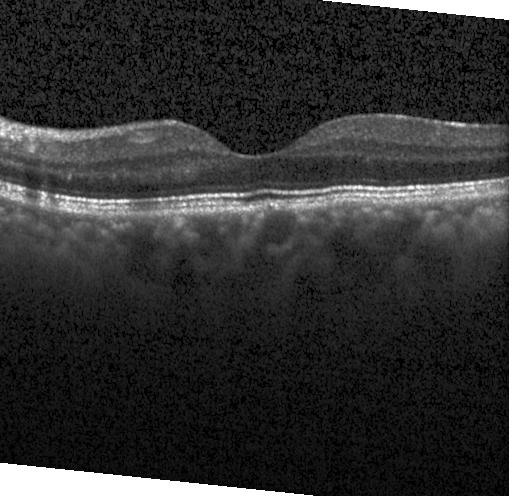

OCT B-scan showing neither CNV, DME, nor drusen.